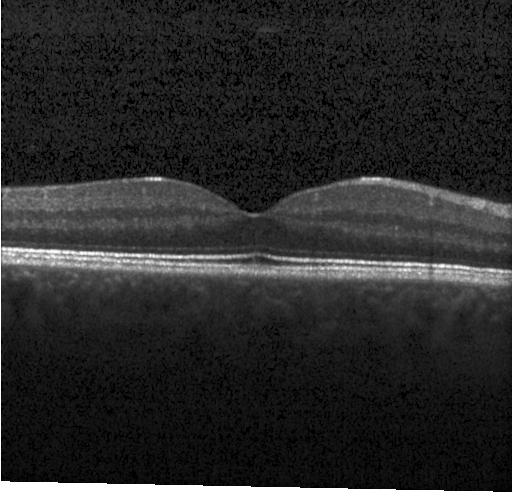
Spectral-domain OCT · retinal OCT B-scan · instrument: Heidelberg Spectralis
Neither CNV, DME, nor drusen.